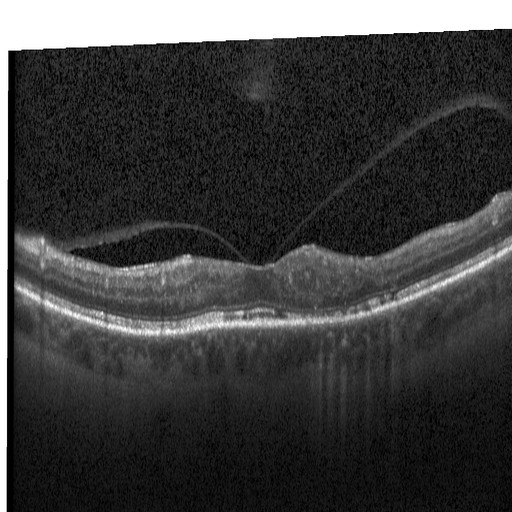

Optical coherence tomography B-scan · spectral-domain OCT.
The scan shows diabetic macular edema.